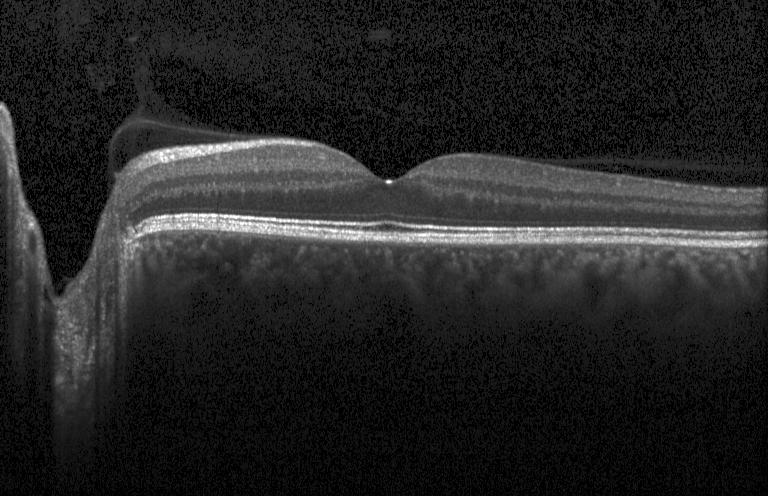
Heidelberg Spectralis OCT system. Macular scan. Retinal OCT B-scan. The scan shows no CNV, DME, or drusen.